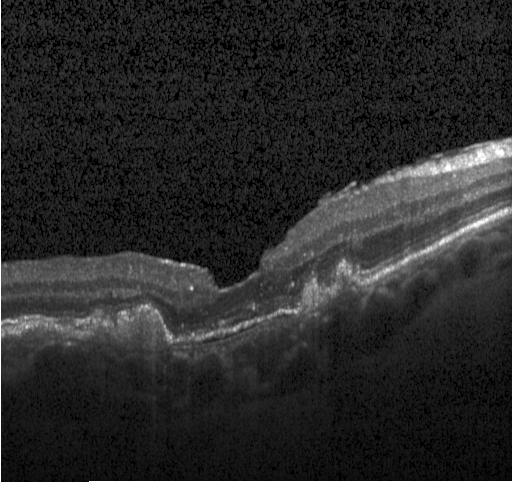
OCT line scan.
Macular OCT: choroidal neovascularization.